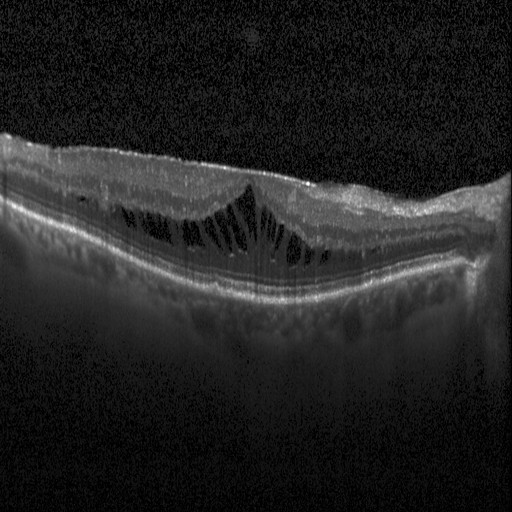
Macular OCT demonstrating diabetic macular edema.